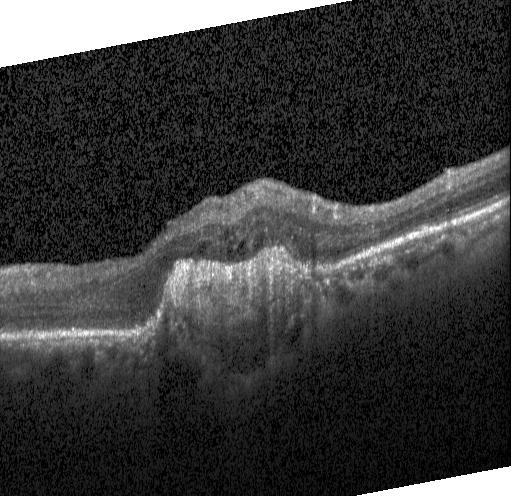
OCT line scan. Centered on the fovea — The scan shows a choroidal neovascular membrane.